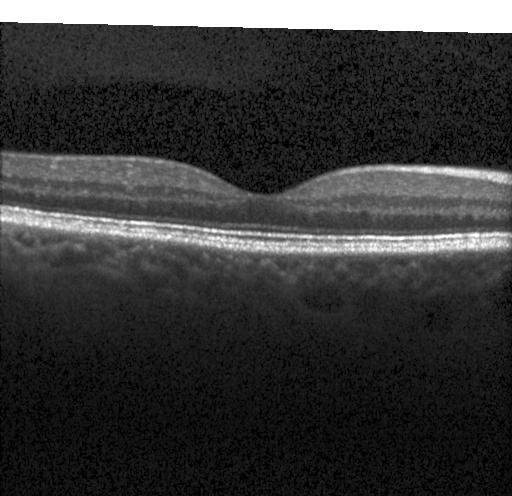 This B-scan demonstrates no choroidal neovascularization, no diabetic macular edema, and no drusen.